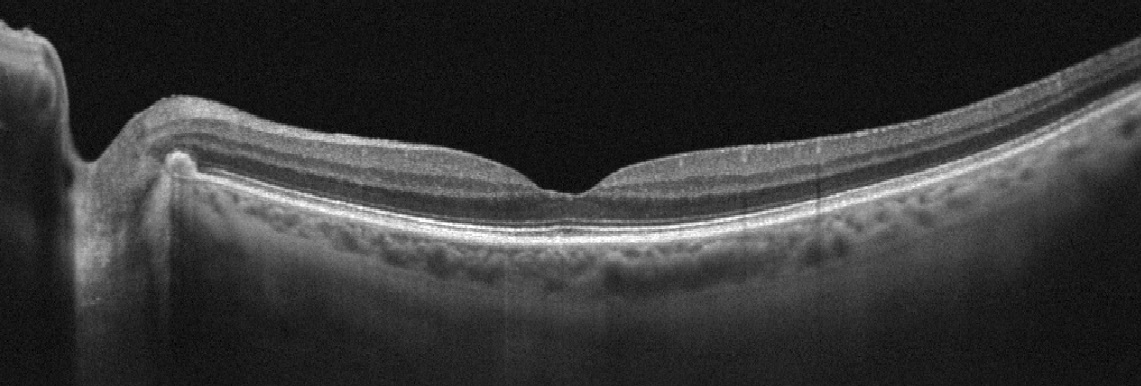 Optical coherence tomography B-scan; instrument: Optovue Avanti RTVue XR.
OCT finding: age-related macular degeneration (AMD).